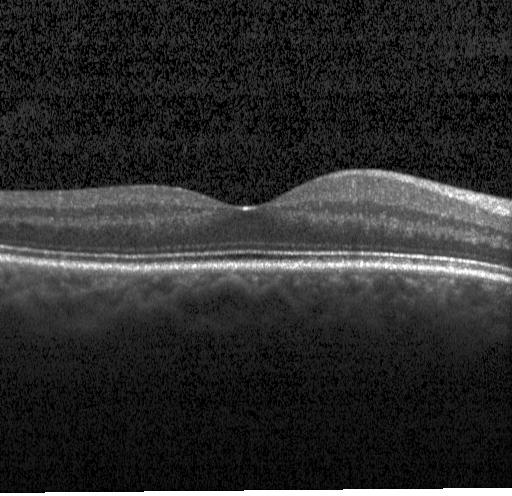
Finding: neither CNV, DME, nor drusen.